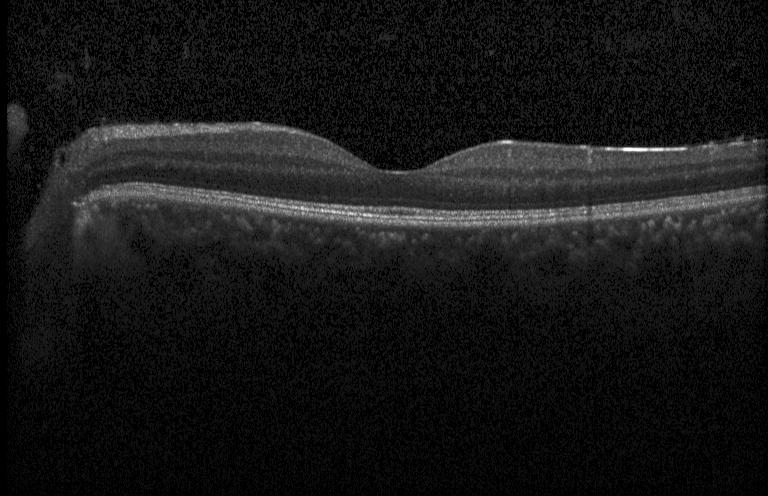
Instrument: Heidelberg Spectralis, spectral-domain OCT, OCT B-scan.
OCT finding: no evidence of choroidal neovascularization, diabetic macular edema, or drusen.